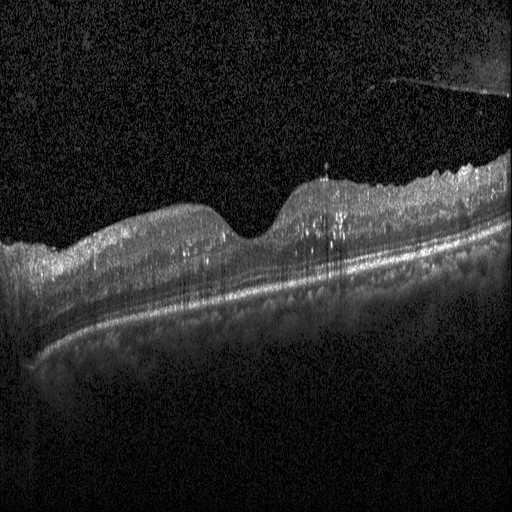

Heidelberg Spectralis. Retinal OCT B-scan. Centered on the fovea. Dx: DME.